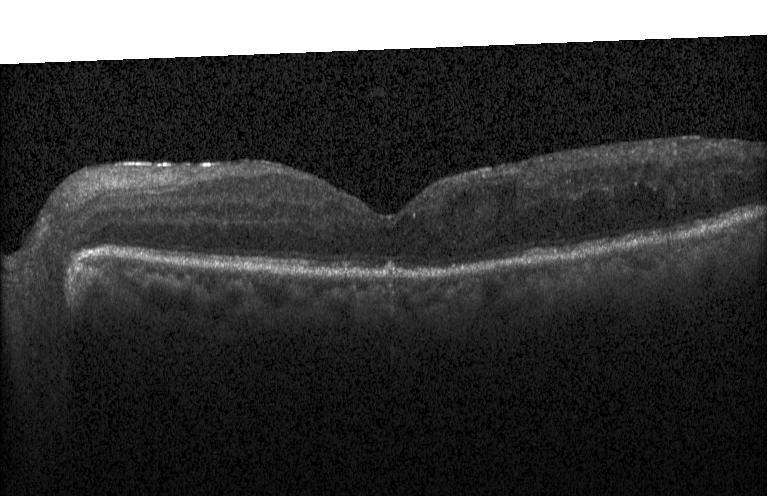

Retinal OCT cross-section showing diabetic macular edema.